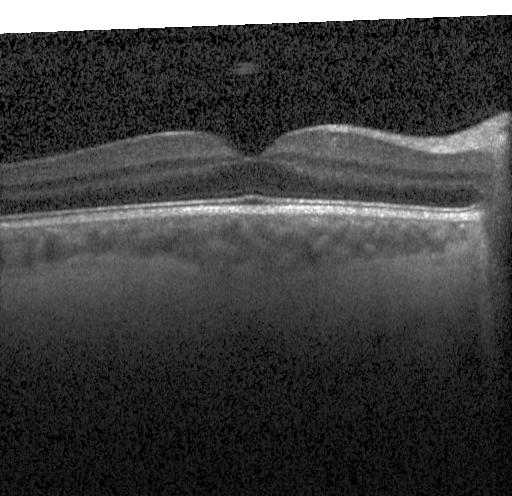

The scan shows no choroidal neovascularization, diabetic macular edema, or drusen.